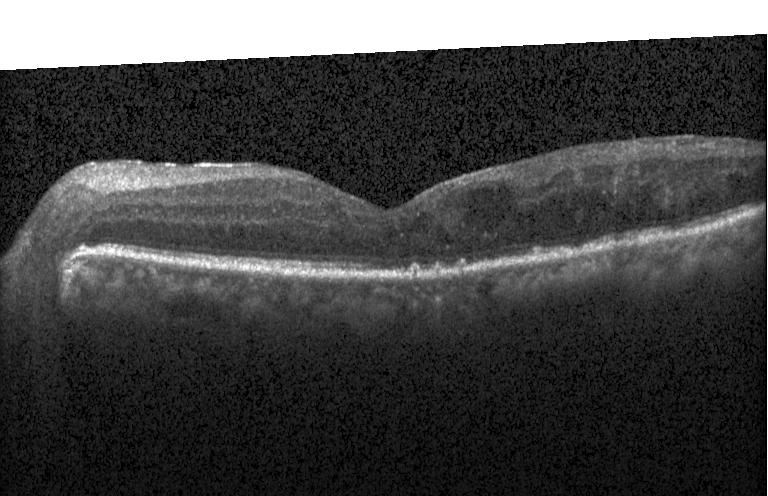
Diagnosis: DME.